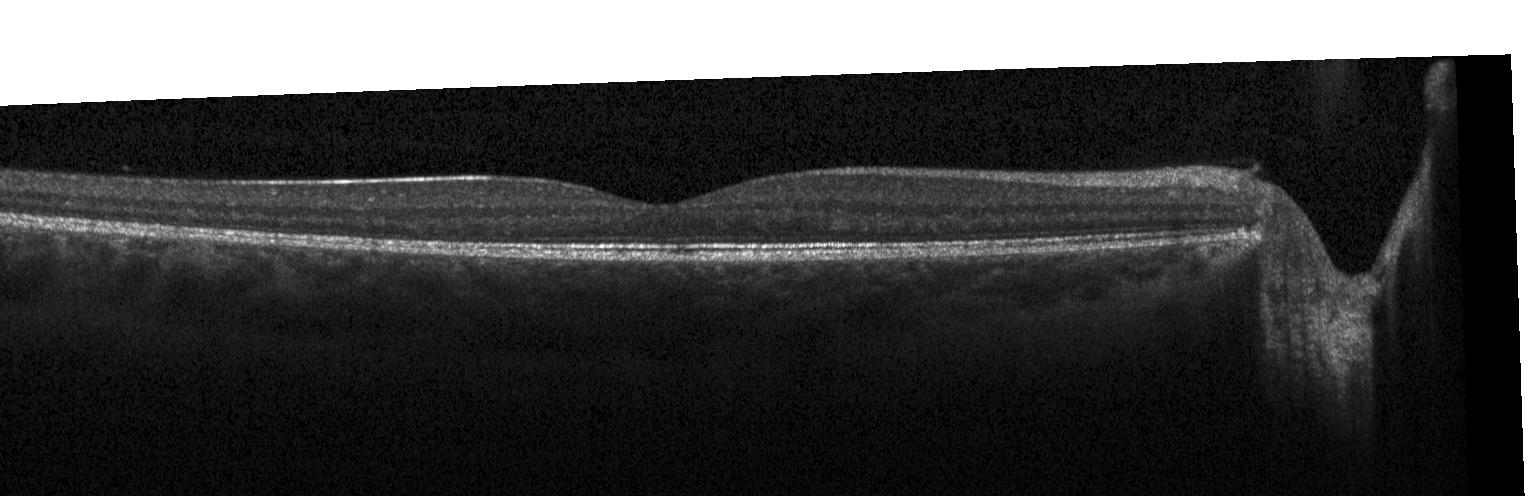

Retinal OCT B-scan.
OCT finding: no choroidal neovascularization, diabetic macular edema, or drusen.